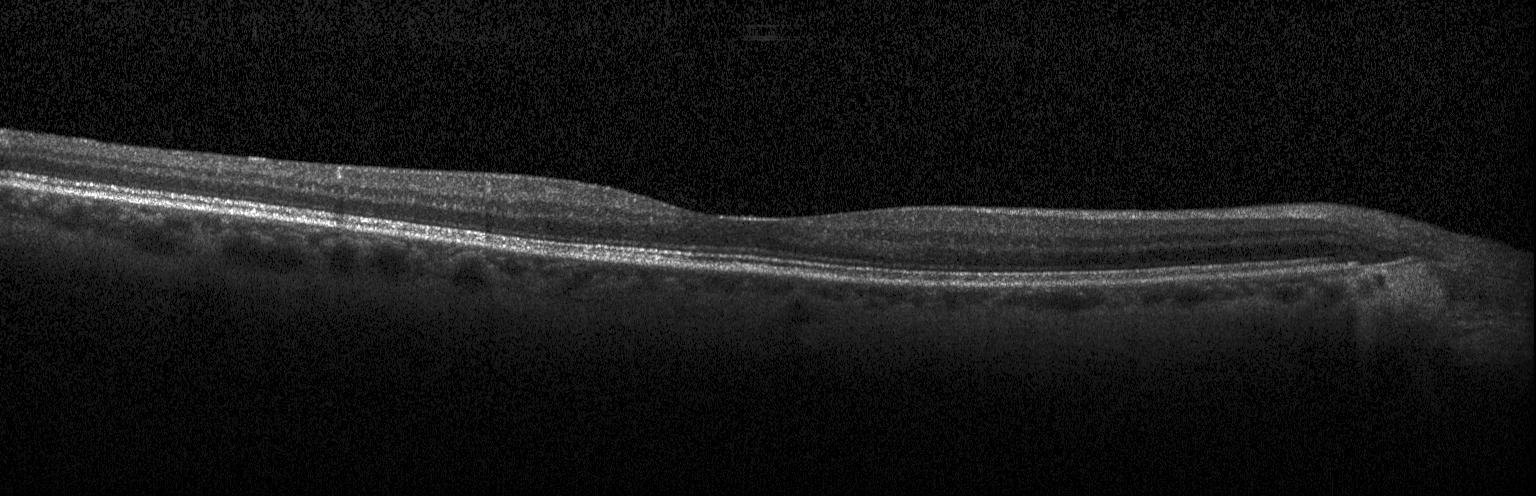
Heidelberg Spectralis OCT system · centered on the fovea · SD-OCT · retinal OCT B-scan — No evidence of CNV, DME, or drusen.